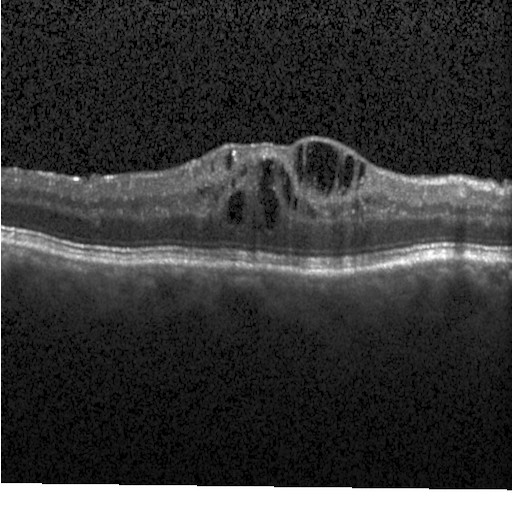
Heidelberg Spectralis; retinal OCT B-scan
OCT finding: DME.